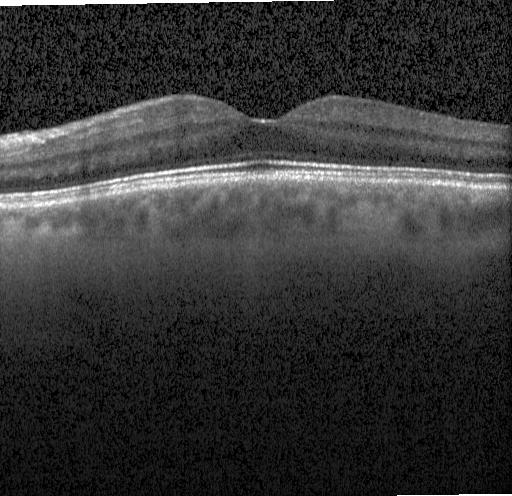

Retinal OCT cross-section; fovea-centered; SD-OCT
Diagnosis: neither choroidal neovascularization, diabetic macular edema, nor drusen.